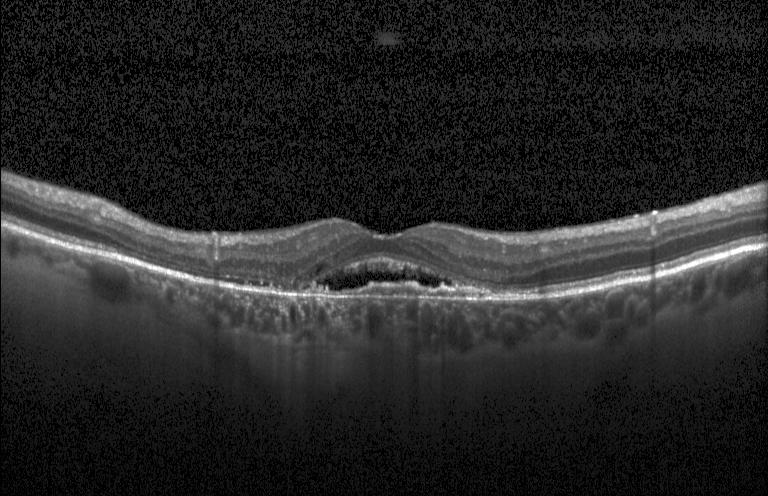

Retinal OCT cross-section, SD-OCT, through the macula, acquired on a Heidelberg Spectralis — Diagnosis: CNV.